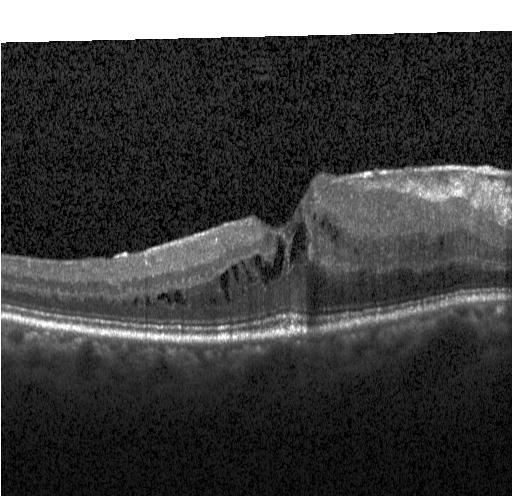 Impression: diabetic macular edema (DME).